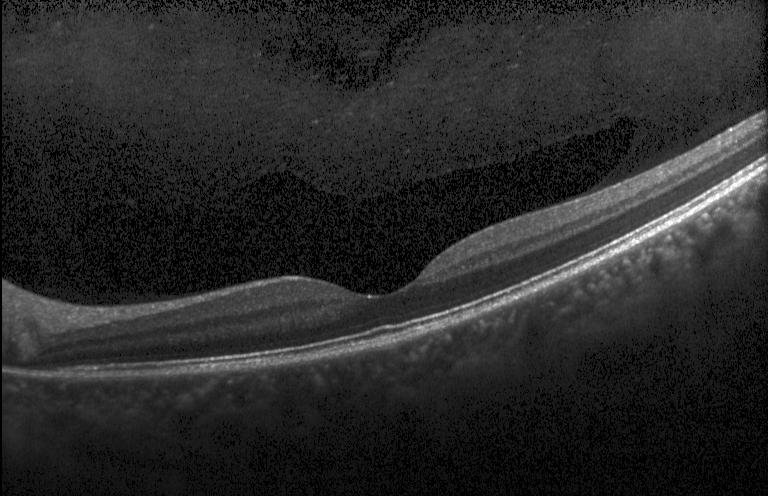

No evidence of CNV, DME, or drusen.